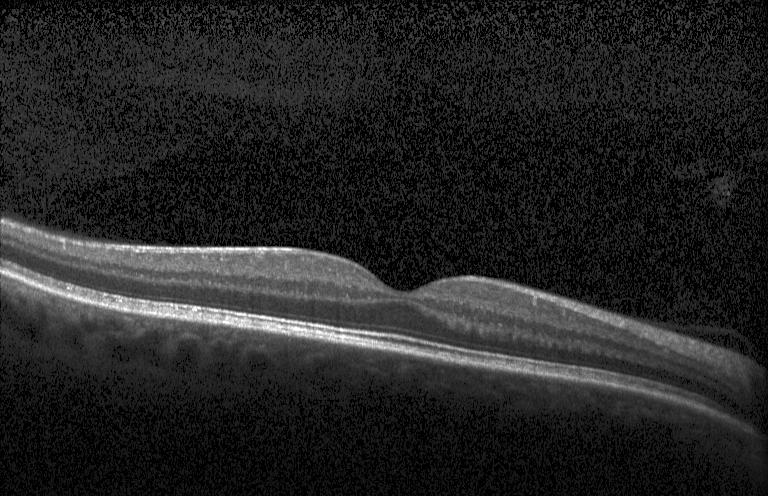 OCT line scan.
Impression: no evidence of choroidal neovascularization, diabetic macular edema, or drusen.